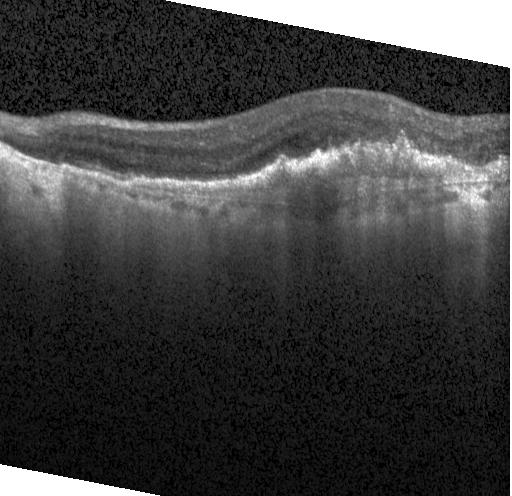
Diagnosis: choroidal neovascularization (CNV).